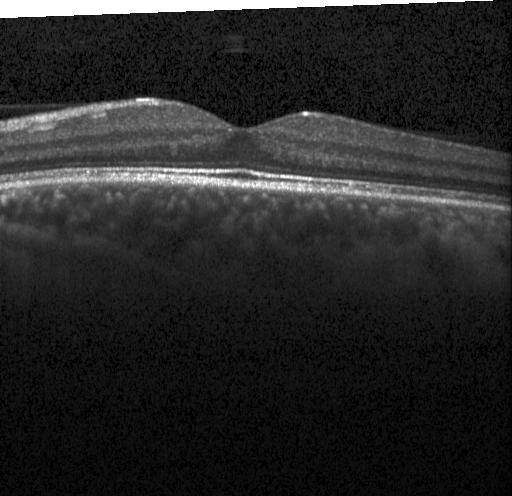

Acquired on a Heidelberg Spectralis, spectral-domain OCT, OCT B-scan
Impression: no choroidal neovascularization, diabetic macular edema, or drusen.